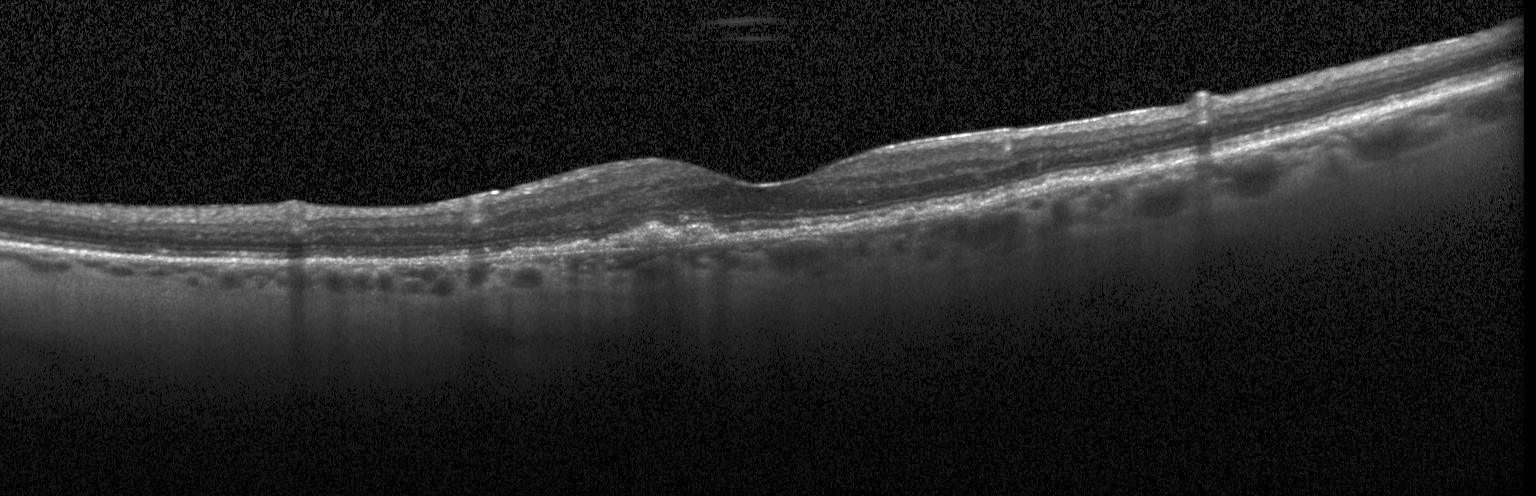
The scan shows choroidal neovascularization (CNV).